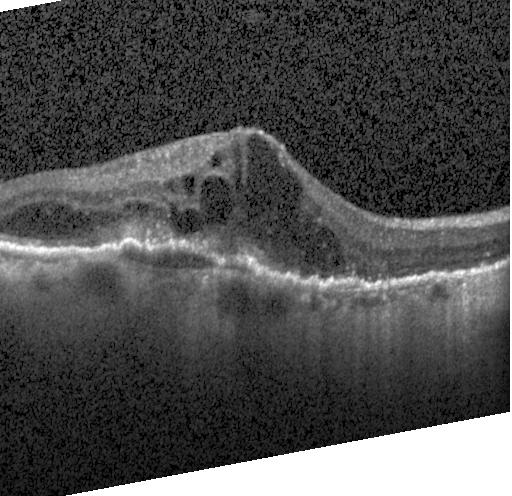

Finding: CNV.